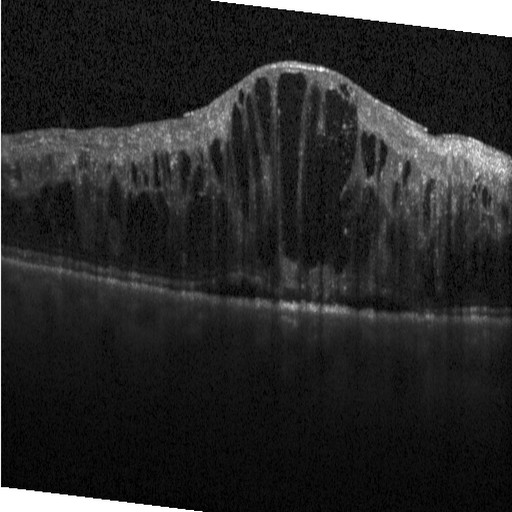
Heidelberg Spectralis OCT system · OCT line scan.
Macular OCT: DME.